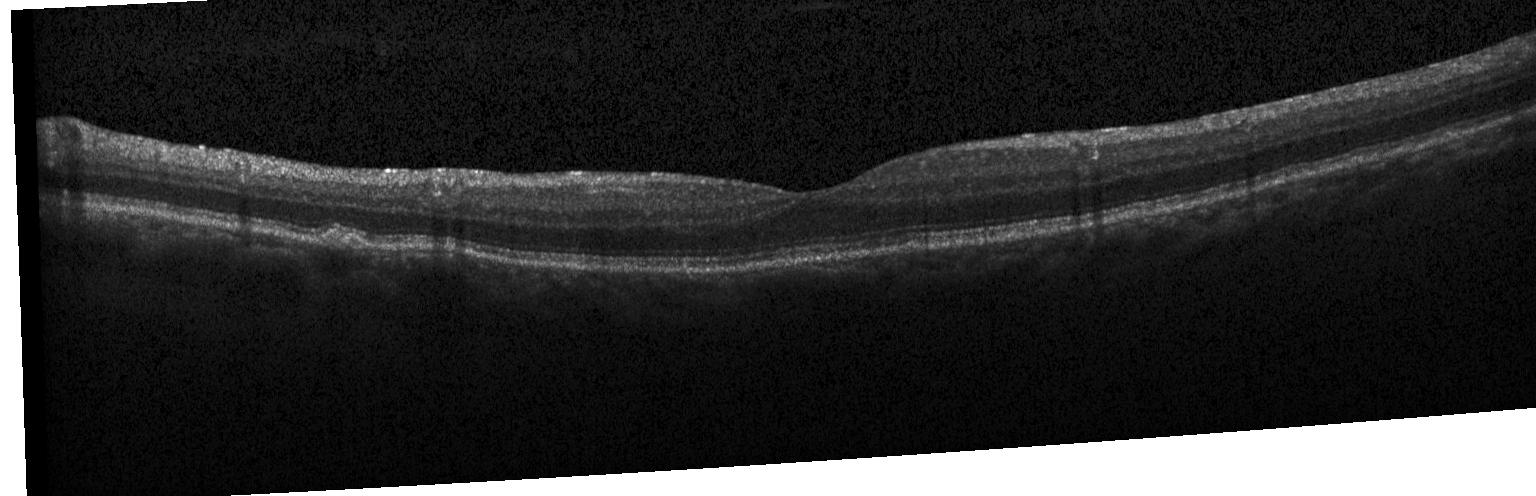 Optical coherence tomography B-scan — The scan shows drusen.